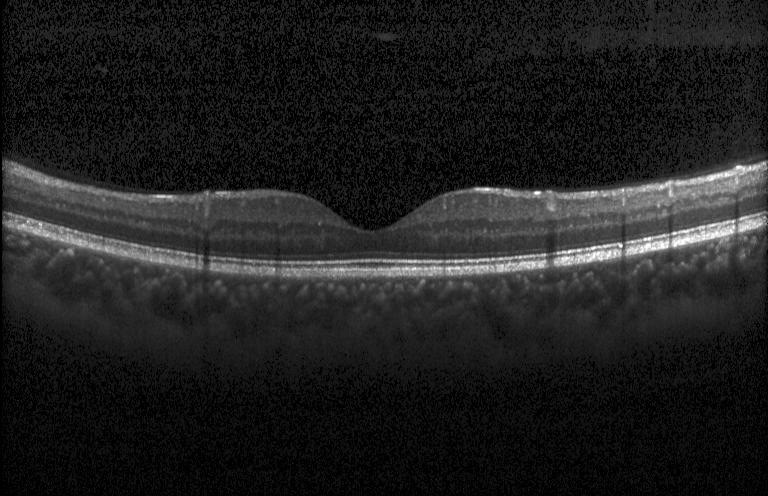

Spectral-domain optical coherence tomography · acquired on a Heidelberg Spectralis · OCT B-scan.
Finding: no choroidal neovascularization, diabetic macular edema, or drusen.